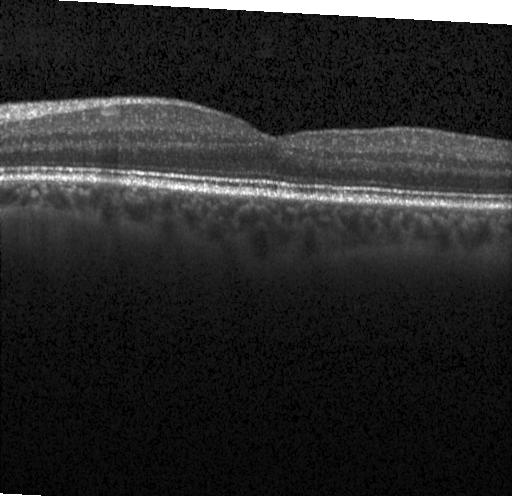

Impression: no evidence of choroidal neovascularization, diabetic macular edema, or drusen.